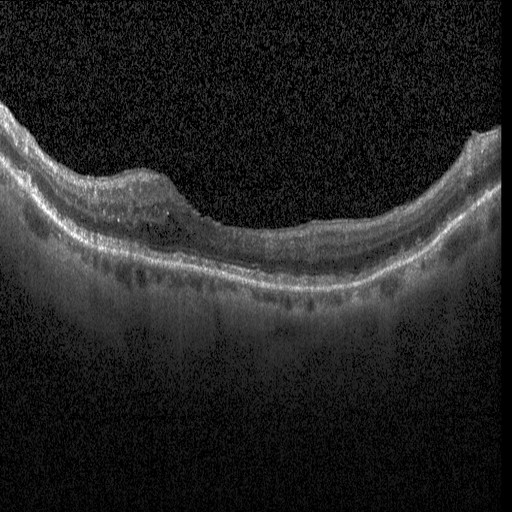 Diagnosis: diabetic macular edema.